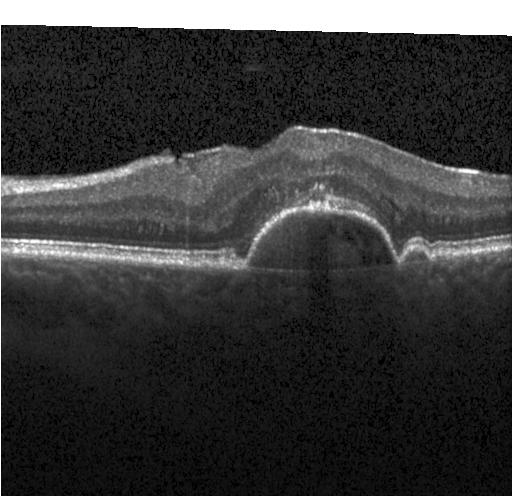

Macular OCT: a choroidal neovascular membrane.